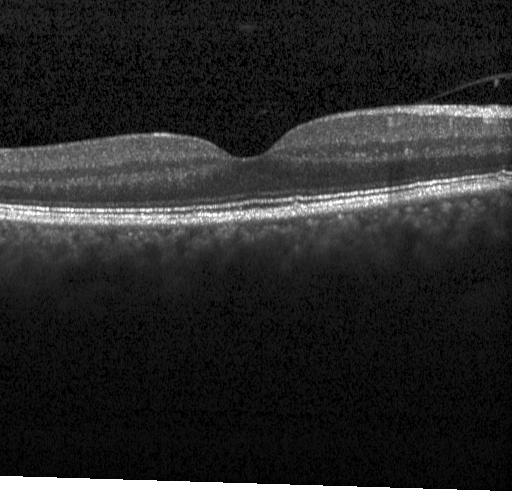

Dx: neither CNV, DME, nor drusen.